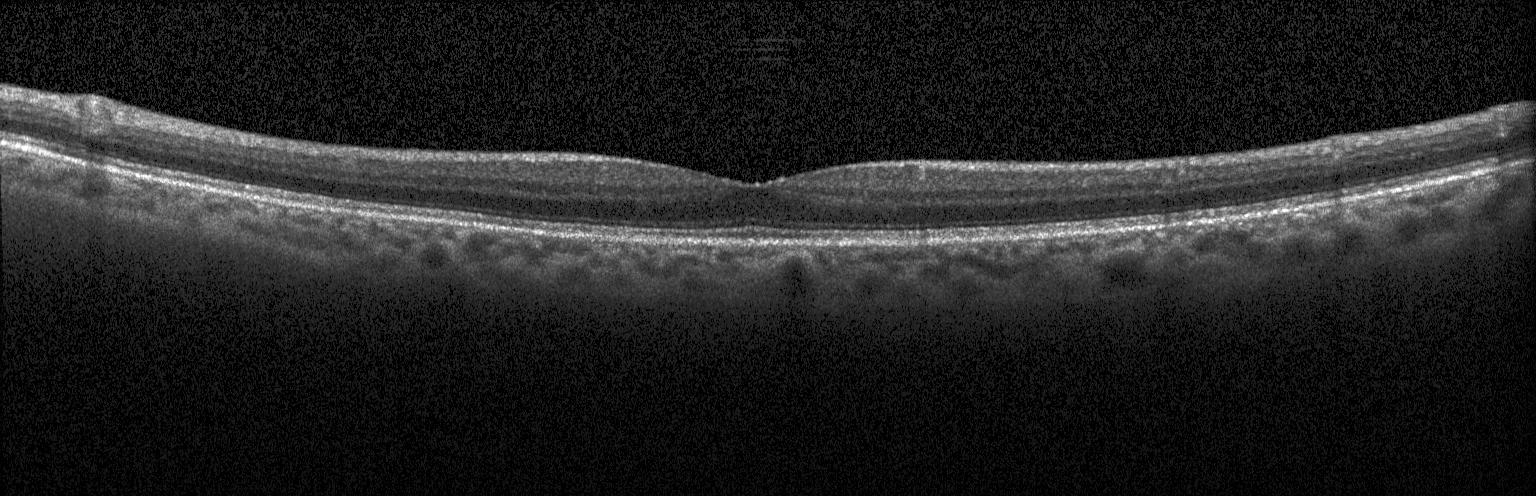
Optical coherence tomography B-scan
Diagnosis: no evidence of CNV, DME, or drusen.